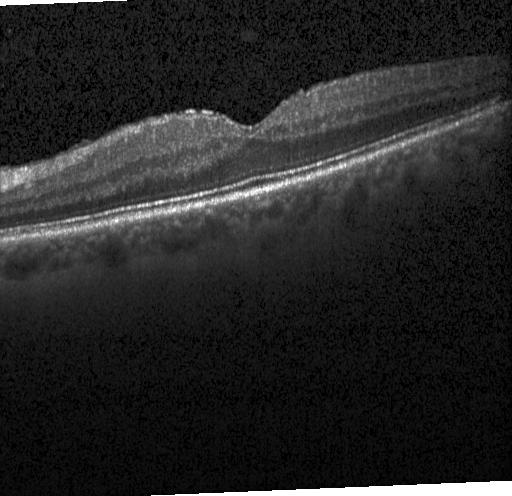

Instrument: Heidelberg Spectralis, macular scan, spectral-domain OCT, OCT B-scan. This B-scan demonstrates neither choroidal neovascularization, diabetic macular edema, nor drusen.